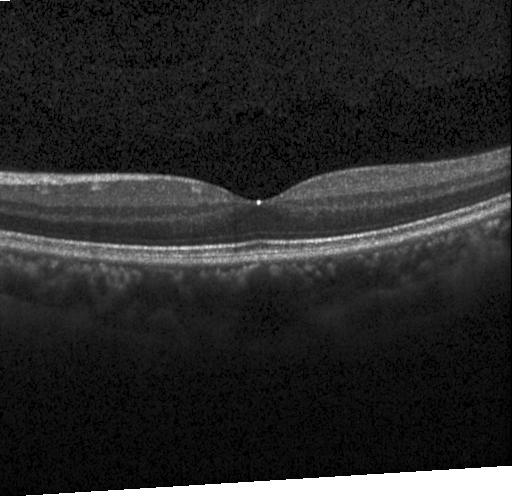
Retinal OCT B-scan.
Diagnosis: neither choroidal neovascularization, diabetic macular edema, nor drusen.